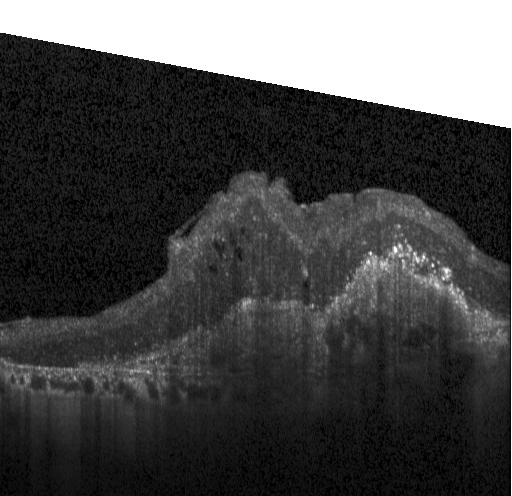

Spectral-domain OCT; retinal OCT B-scan. Finding: a choroidal neovascular membrane.